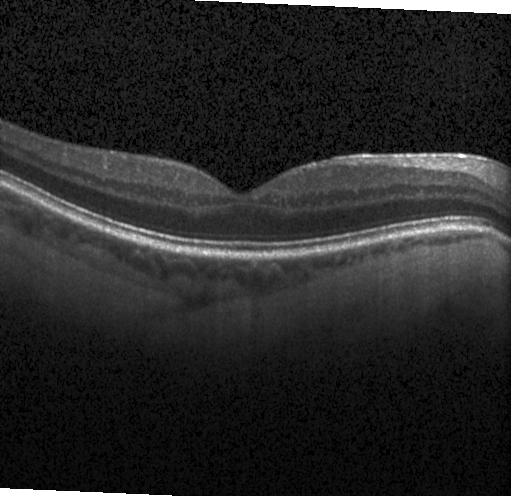

SD-OCT; through the macula; Heidelberg Spectralis; retinal OCT B-scan — Diagnosis: no choroidal neovascularization, no diabetic macular edema, and no drusen.